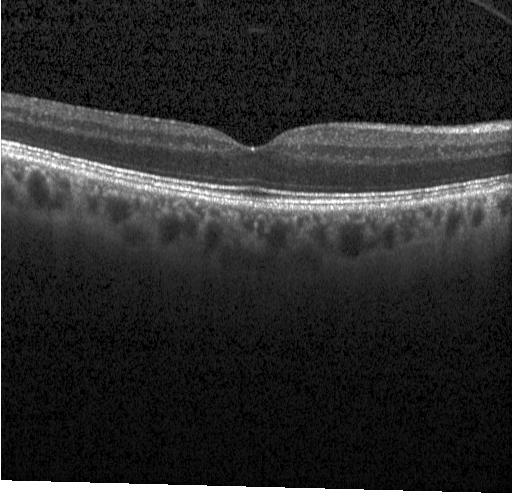

Spectral-domain optical coherence tomography, acquired on a Heidelberg Spectralis, OCT B-scan, horizontal scan through the fovea
Diagnosis: no choroidal neovascularization, diabetic macular edema, or drusen.